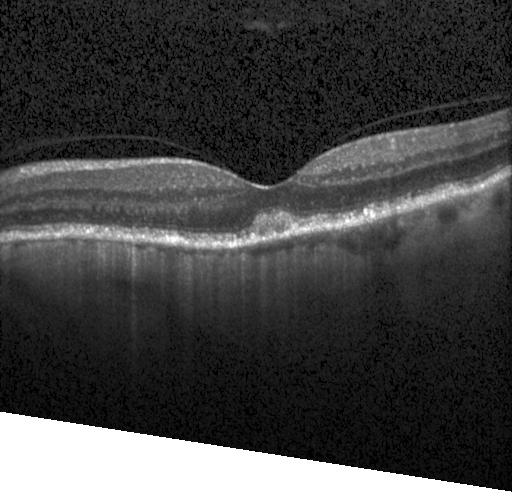
OCT finding: multiple drusen.